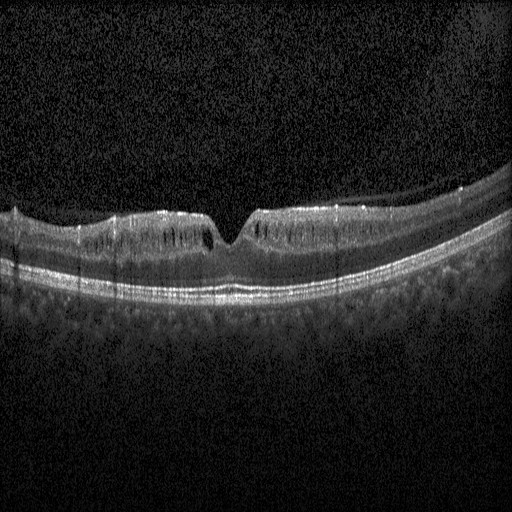 Heidelberg Spectralis OCT system, optical coherence tomography B-scan, SD-OCT. Impression: diabetic macular edema (DME).